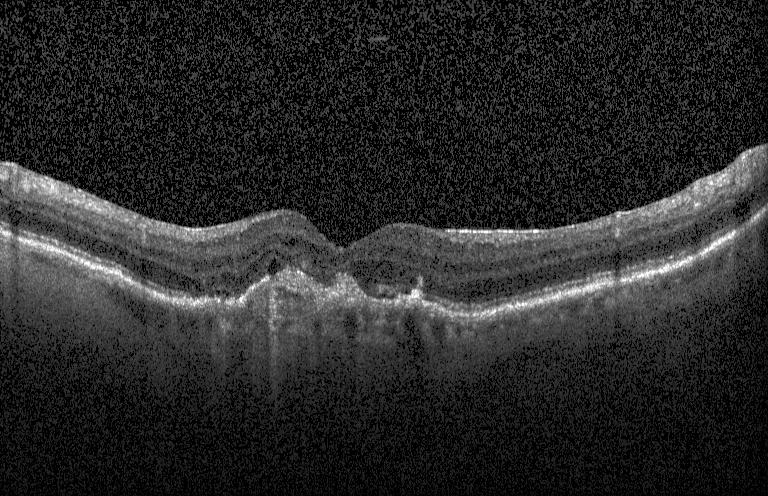
Macular OCT demonstrating a choroidal neovascular membrane.